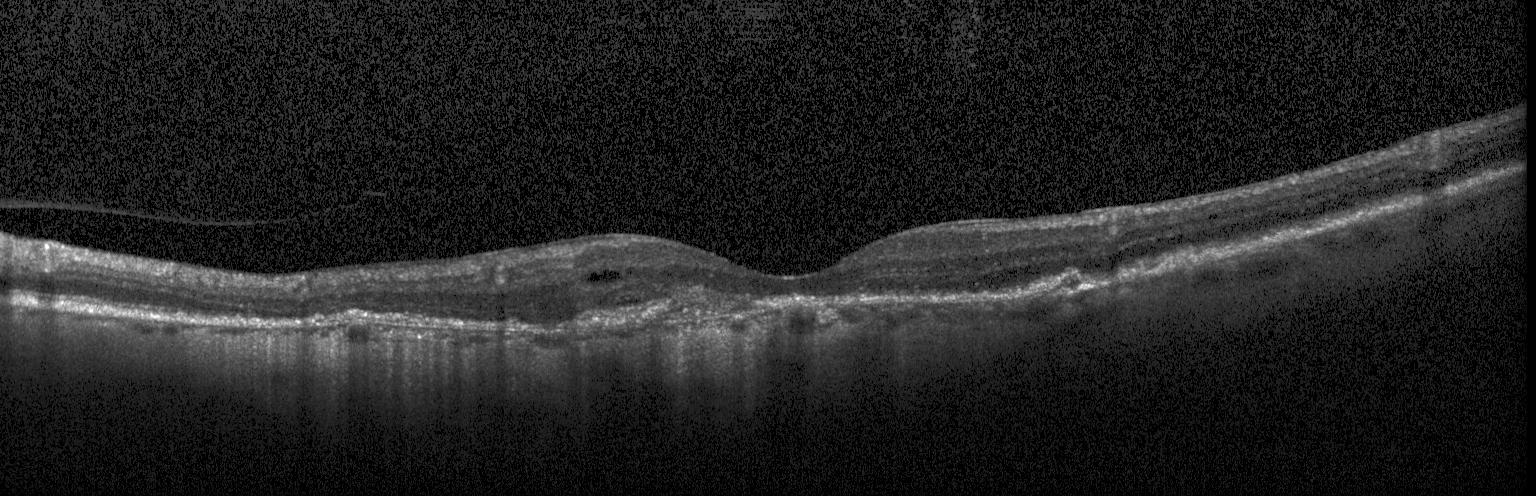

OCT scan showing CNV.